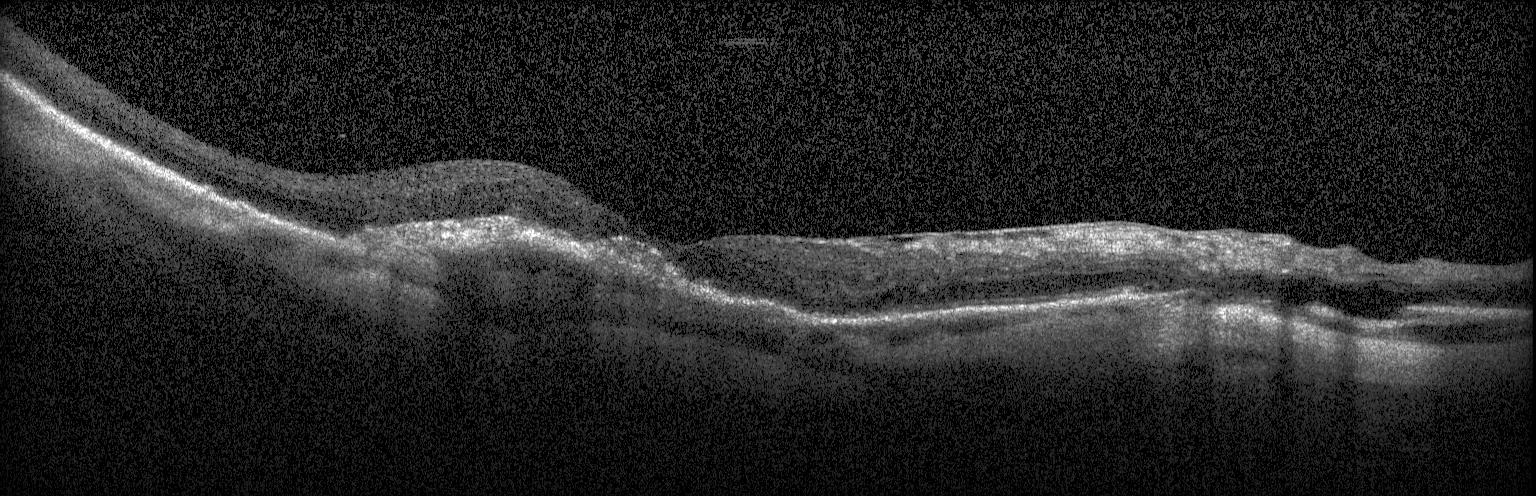
Retinal OCT cross-section
Diagnosis: CNV.